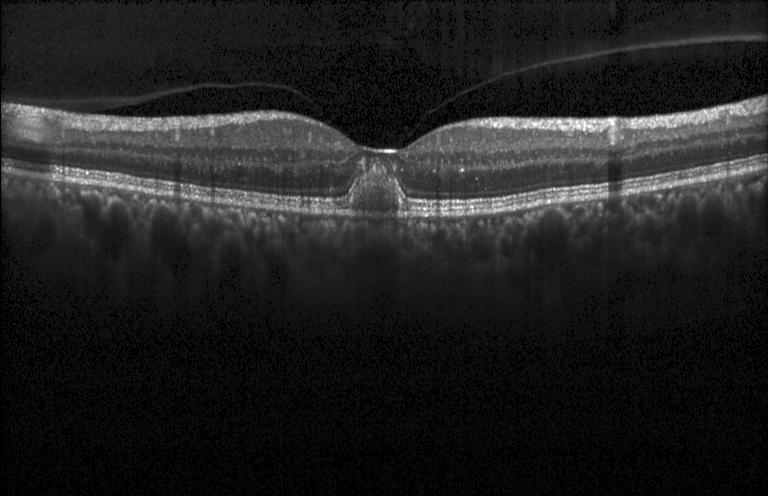

OCT B-scan. Instrument: Heidelberg Spectralis. SD-OCT. Fovea-centered
Diagnosis: a choroidal neovascular membrane.